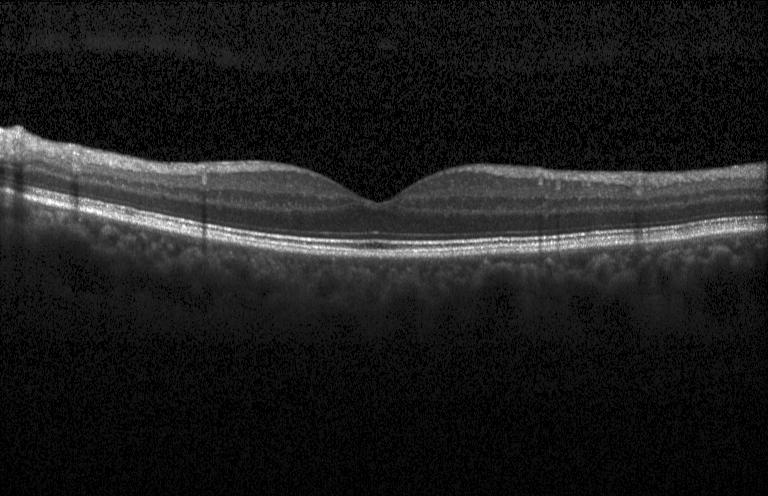

Instrument: Heidelberg Spectralis. SD-OCT. Retinal OCT B-scan. Diagnosis: no choroidal neovascularization, no diabetic macular edema, and no drusen.